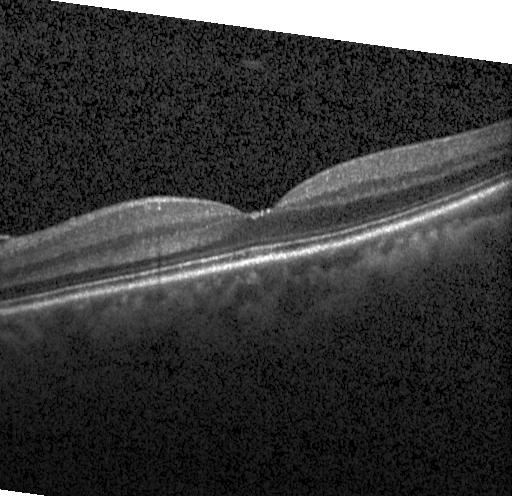
OCT B-scan showing no choroidal neovascularization, diabetic macular edema, or drusen.